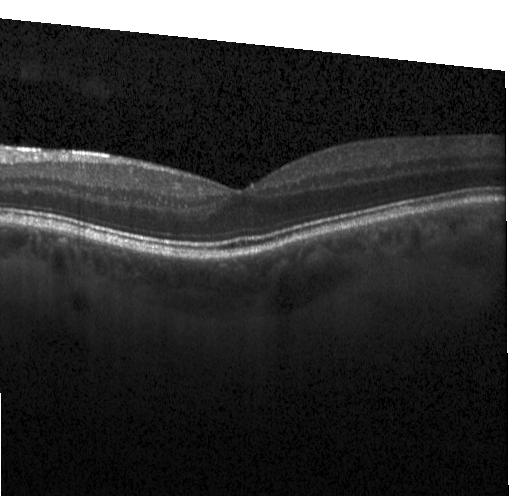 Optical coherence tomography scan · fovea-centered · spectral-domain OCT — Impression: no choroidal neovascularization, diabetic macular edema, or drusen.